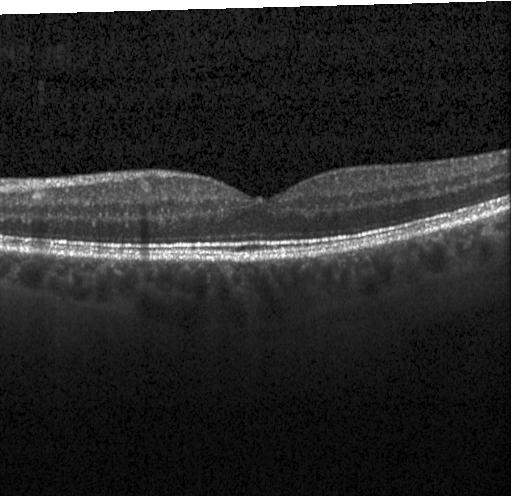 Spectral-domain optical coherence tomography. OCT B-scan. Acquired on a Heidelberg Spectralis — Diagnosis: no choroidal neovascularization, diabetic macular edema, or drusen.